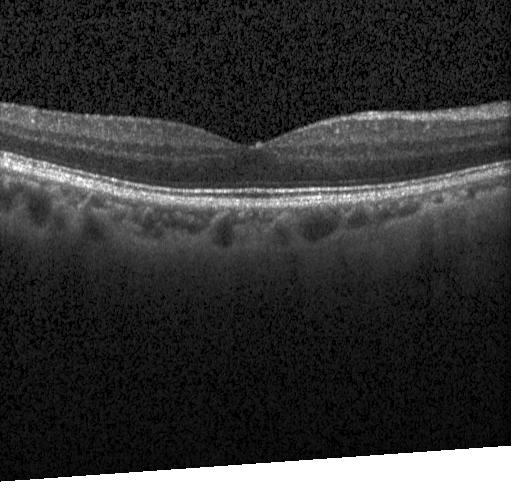
The scan shows neither choroidal neovascularization, diabetic macular edema, nor drusen.